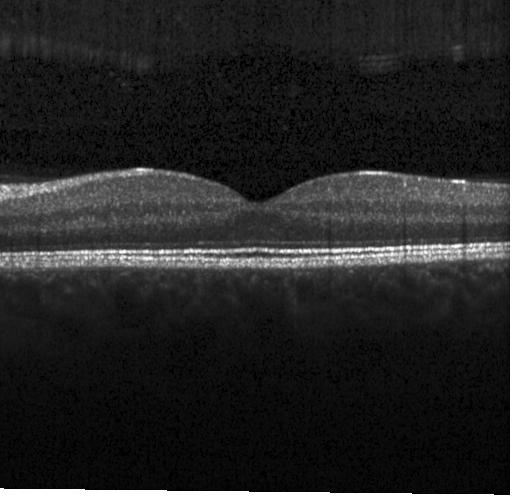 Heidelberg Spectralis OCT system · fovea-centered · retinal OCT B-scan · spectral-domain optical coherence tomography.
Finding: no CNV, no DME, and no drusen.